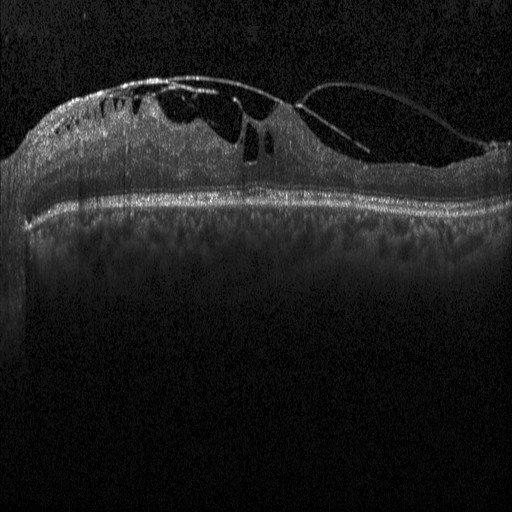
Heidelberg Spectralis OCT system, retinal OCT cross-section, SD-OCT. Assessment: diabetic macular edema (DME).